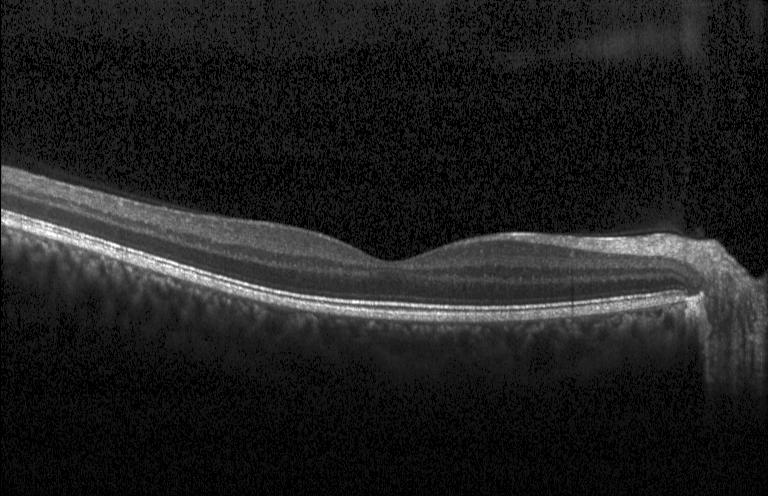

Diagnosis: neither choroidal neovascularization, diabetic macular edema, nor drusen.